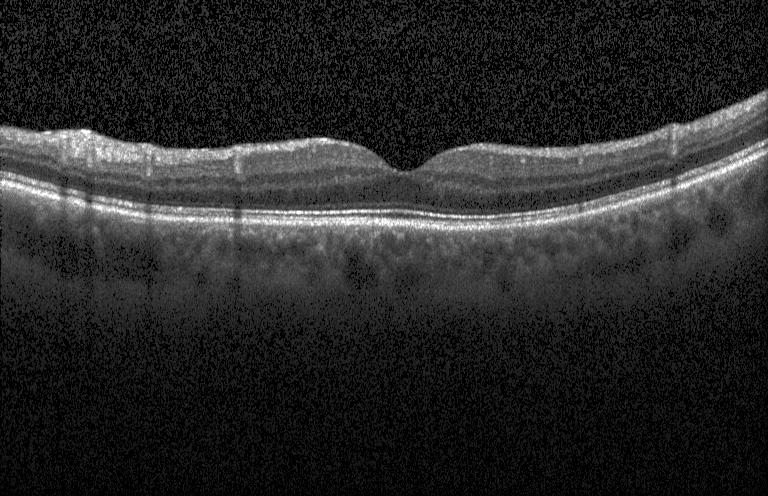

Macular OCT demonstrating no evidence of CNV, DME, or drusen.